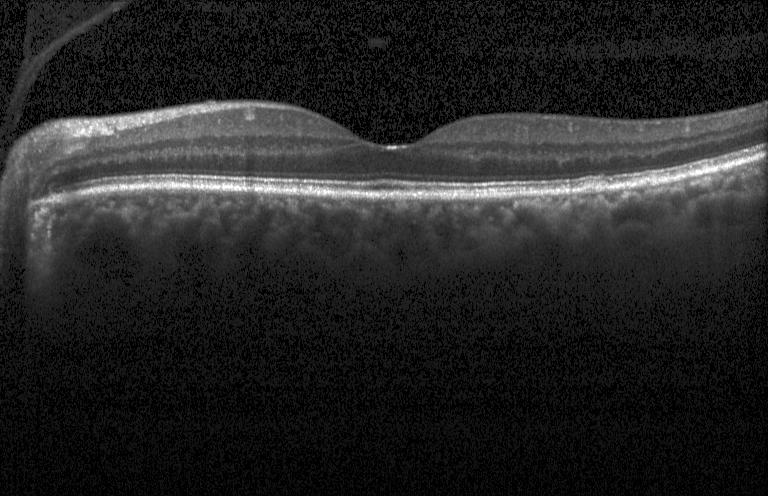 Retinal OCT B-scan.
Dx: no CNV, no DME, and no drusen.